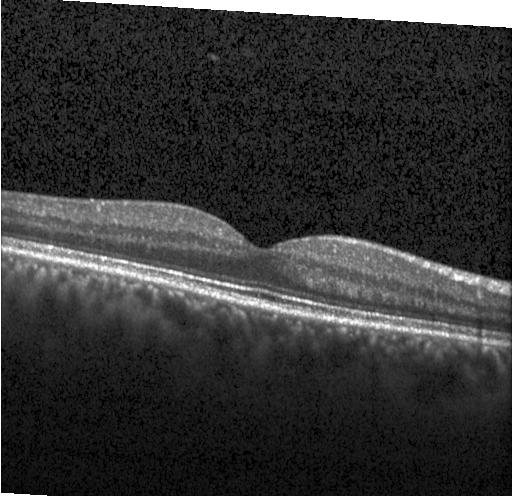

Horizontal scan through the fovea, retinal OCT cross-section, Heidelberg Spectralis OCT system
Finding: neither CNV, DME, nor drusen.